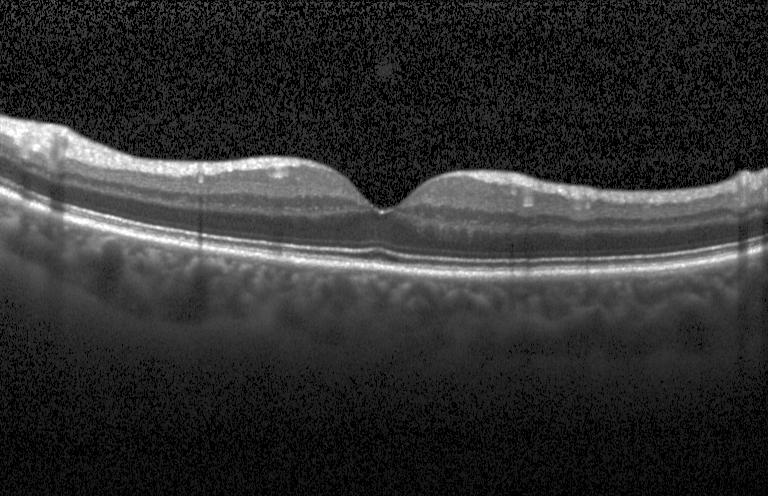 Instrument: Heidelberg Spectralis; retinal OCT B-scan; macular scan; spectral-domain OCT — Assessment: no evidence of choroidal neovascularization, diabetic macular edema, or drusen.